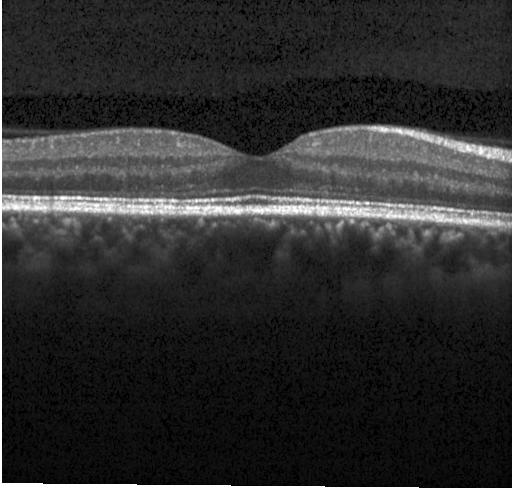
OCT line scan; through the macula. Assessment: neither CNV, DME, nor drusen.